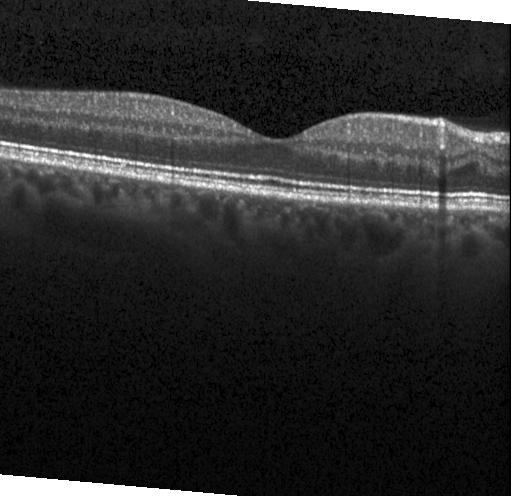
SD-OCT. Retinal OCT B-scan — Finding: no choroidal neovascularization, diabetic macular edema, or drusen.